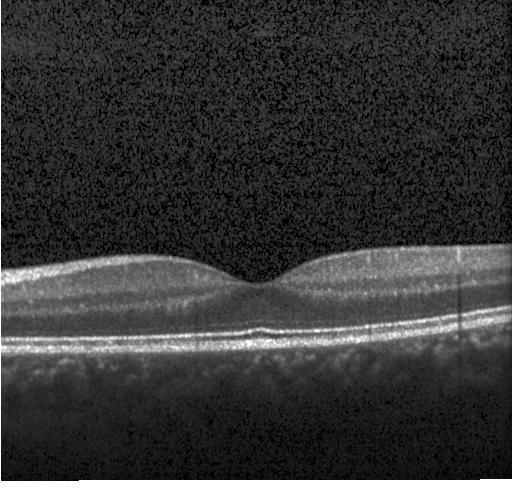 Spectral-domain OCT · optical coherence tomography B-scan. Dx: neither CNV, DME, nor drusen.